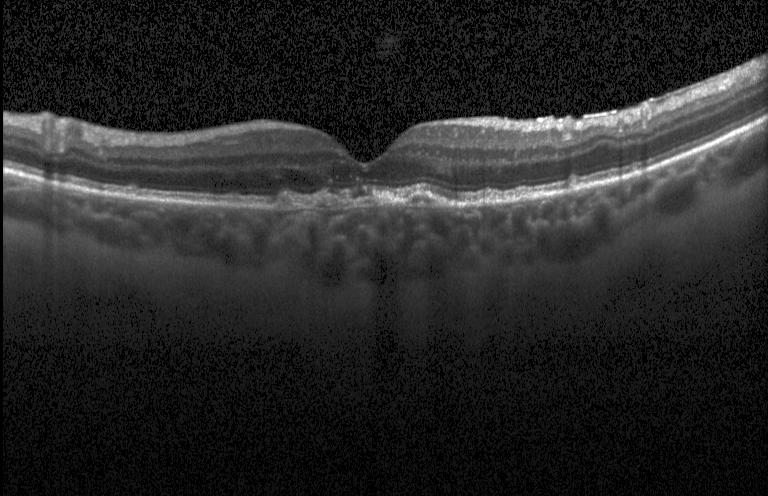 OCT line scan
Impression: a choroidal neovascular membrane.